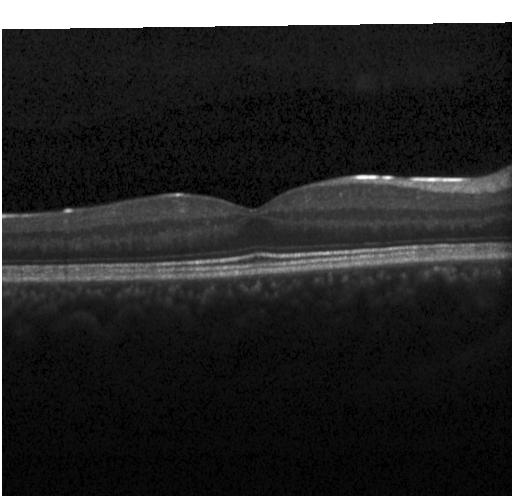

Retinal OCT cross-section; Heidelberg Spectralis — Impression: neither choroidal neovascularization, diabetic macular edema, nor drusen.